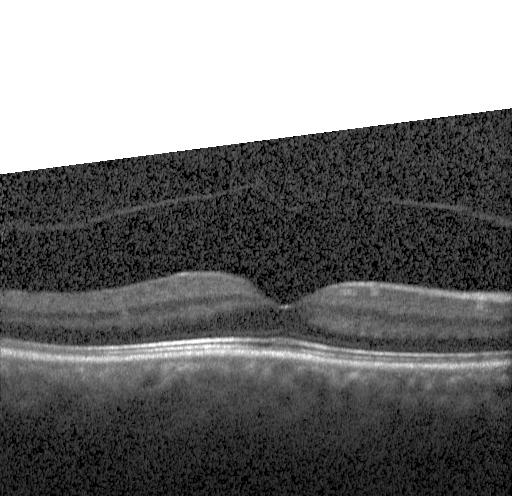 Finding: neither CNV, DME, nor drusen.